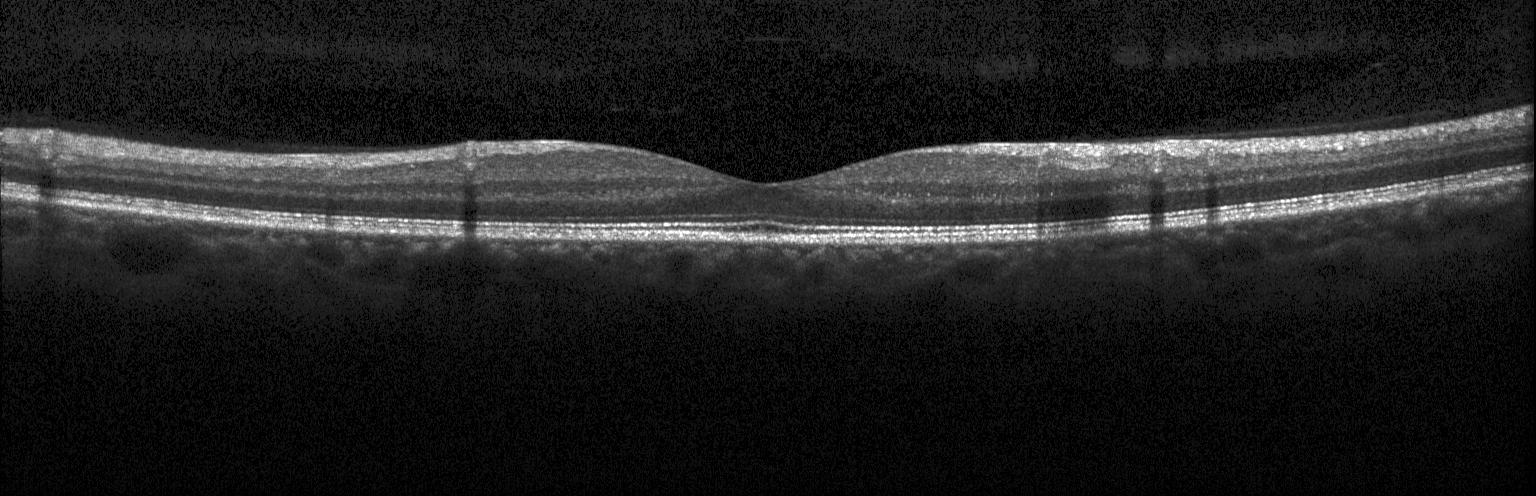
Horizontal scan through the fovea · Heidelberg Spectralis · OCT B-scan — Impression: no choroidal neovascularization, diabetic macular edema, or drusen.